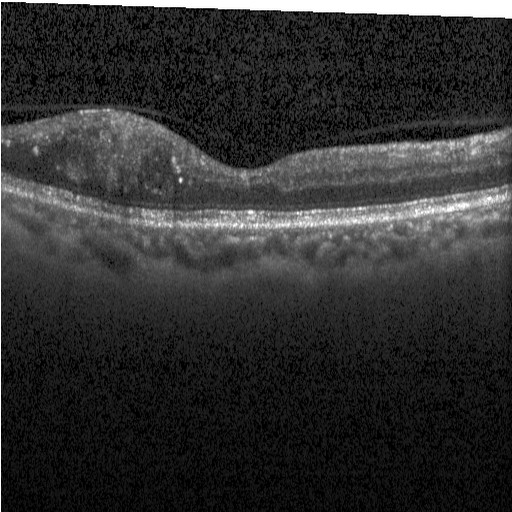

Finding: DME.